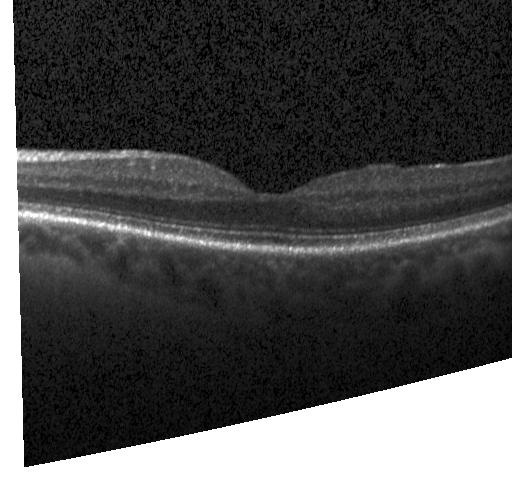 Fovea-centered · retinal OCT cross-section · instrument: Heidelberg Spectralis · spectral-domain OCT. Diagnosis: no choroidal neovascularization, diabetic macular edema, or drusen.